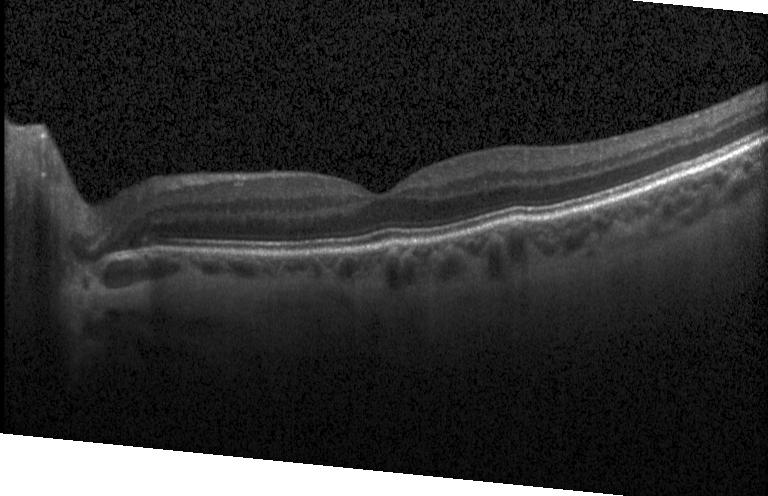 OCT line scan · macular scan — The scan shows neither CNV, DME, nor drusen.